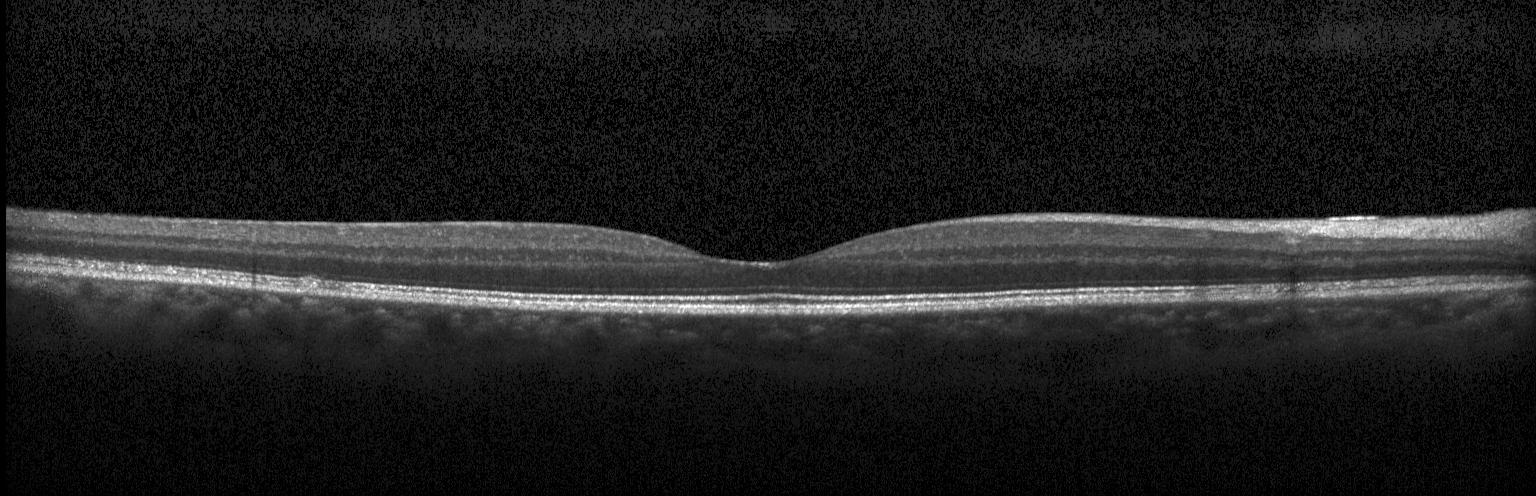
Diagnosis: no choroidal neovascularization, diabetic macular edema, or drusen.